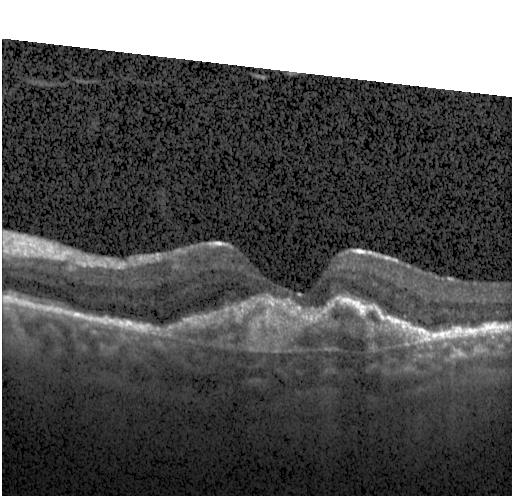

SD-OCT, retinal OCT B-scan. Diagnosis: a choroidal neovascular membrane.